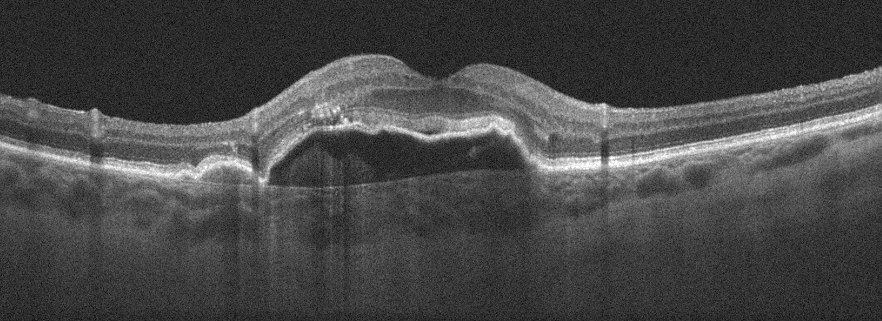 OCT B-scan · right eye — The scan shows age-related macular degeneration.